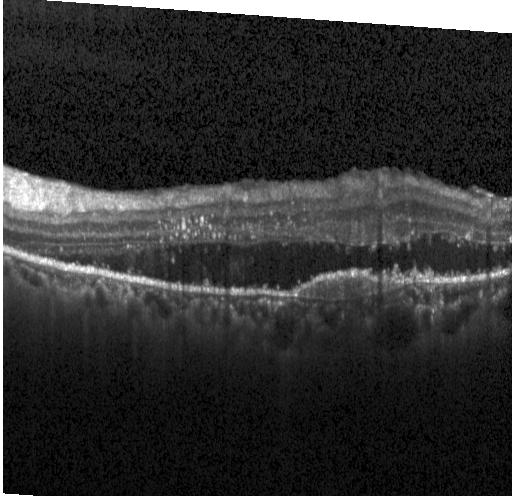
OCT B-scan.
Choroidal neovascularization.